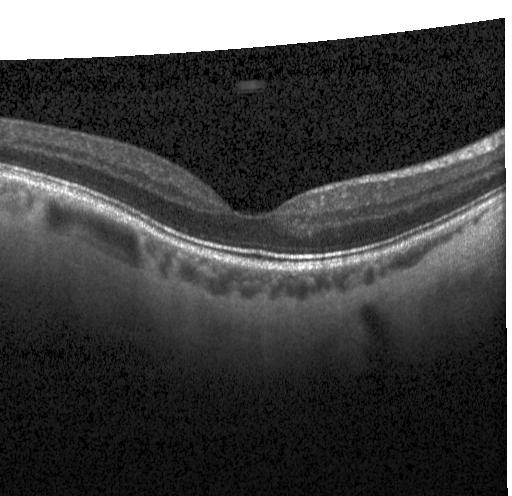 Spectral-domain OCT B-scan: no CNV, DME, or drusen.